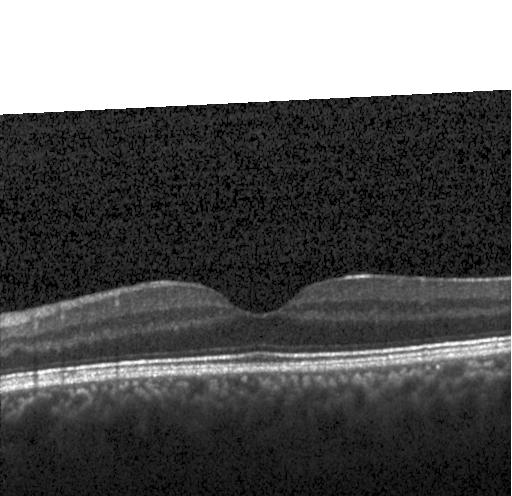
OCT B-scan · centered on the fovea. The scan shows no choroidal neovascularization, diabetic macular edema, or drusen.